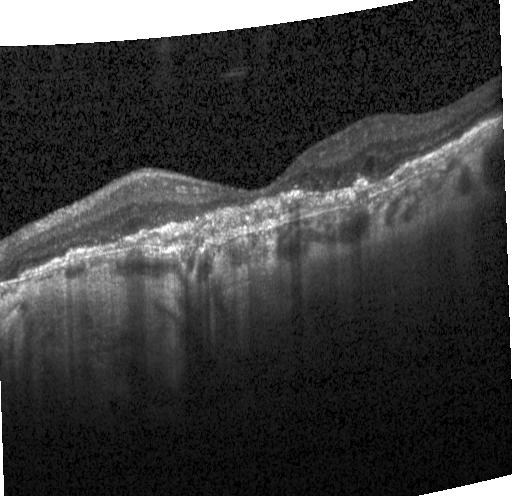 Heidelberg Spectralis; horizontal scan through the fovea; OCT B-scan
Diagnosis: choroidal neovascularization (CNV).